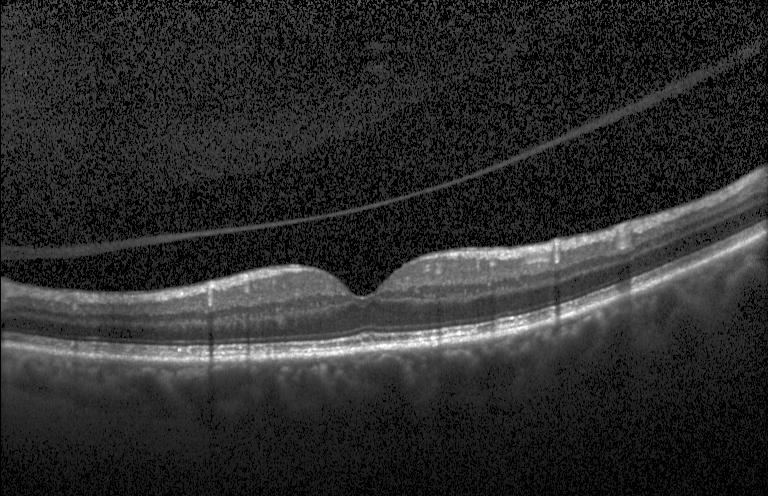 Acquired on a Heidelberg Spectralis. Centered on the fovea. OCT B-scan — No choroidal neovascularization, no diabetic macular edema, and no drusen.